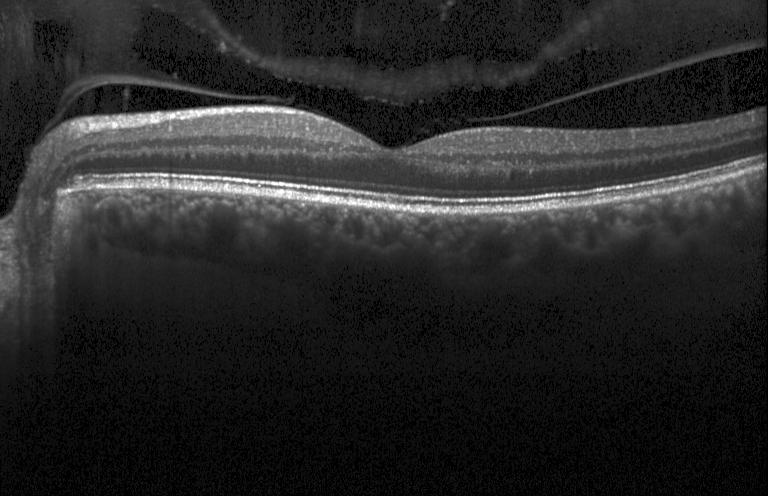 Horizontal scan through the fovea; spectral-domain OCT; OCT line scan; instrument: Heidelberg Spectralis
Diagnosis: no CNV, no DME, and no drusen.